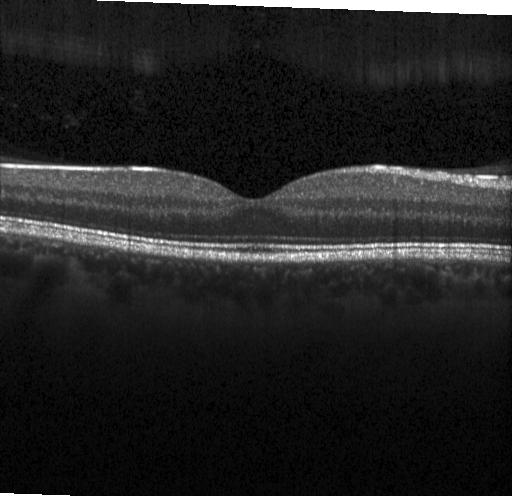
Macular OCT: no evidence of choroidal neovascularization, diabetic macular edema, or drusen.